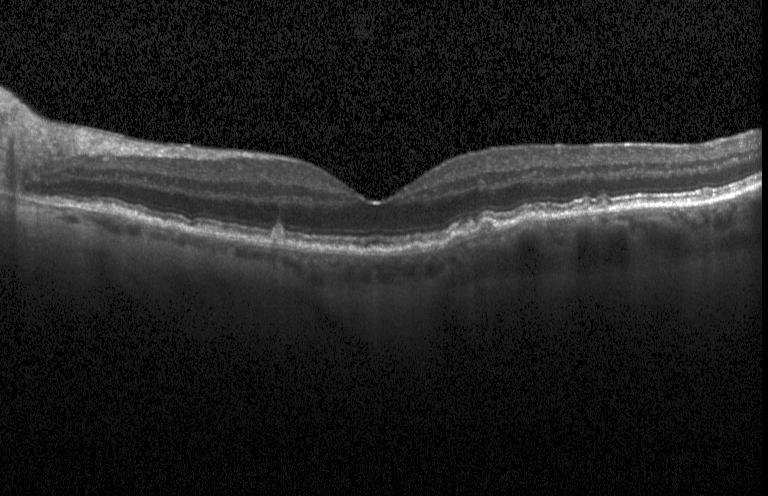

Optical coherence tomography B-scan — Finding: multiple drusen.